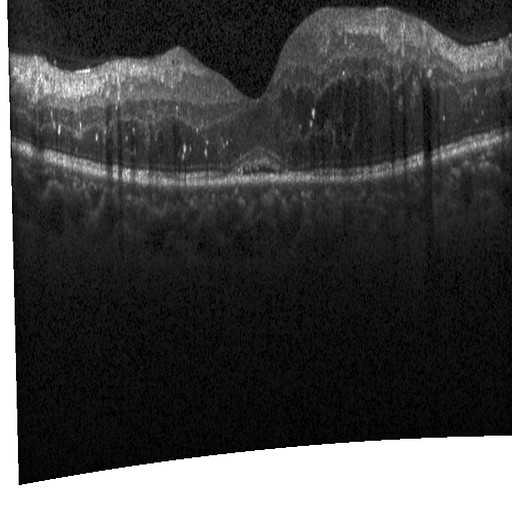 Heidelberg Spectralis · spectral-domain optical coherence tomography · through the macula · OCT line scan. Diabetic macular edema.